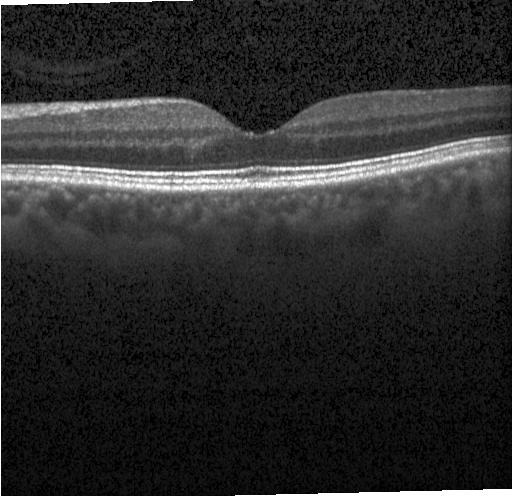
Retinal OCT cross-section.
Diagnosis: no evidence of CNV, DME, or drusen.